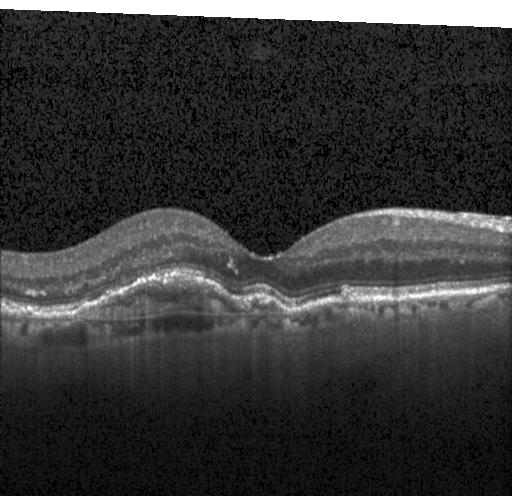

Optical coherence tomography scan, Heidelberg Spectralis.
Diagnosis: a choroidal neovascular membrane.